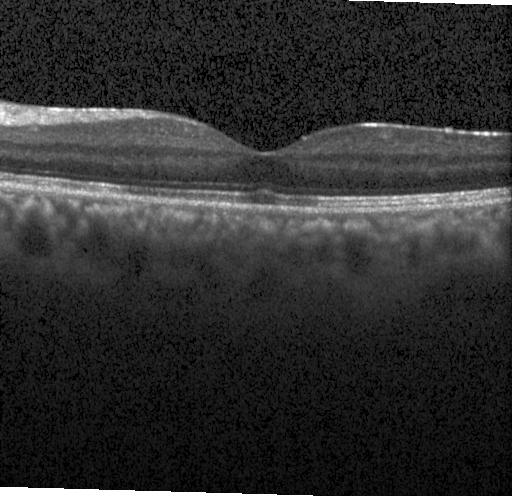

Optical coherence tomography B-scan.
Impression: no evidence of CNV, DME, or drusen.